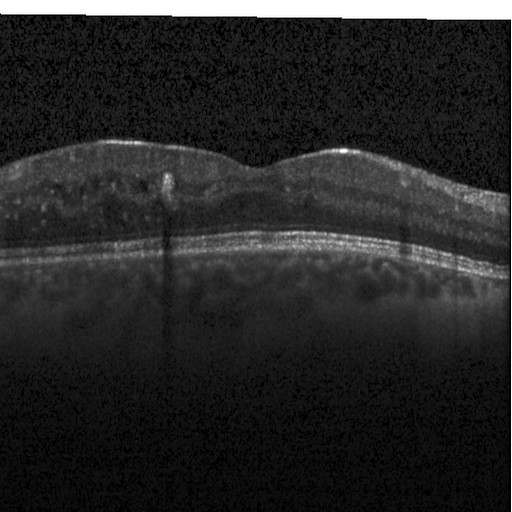 OCT line scan · Heidelberg Spectralis · through the macula · SD-OCT. Impression: diabetic macular edema.